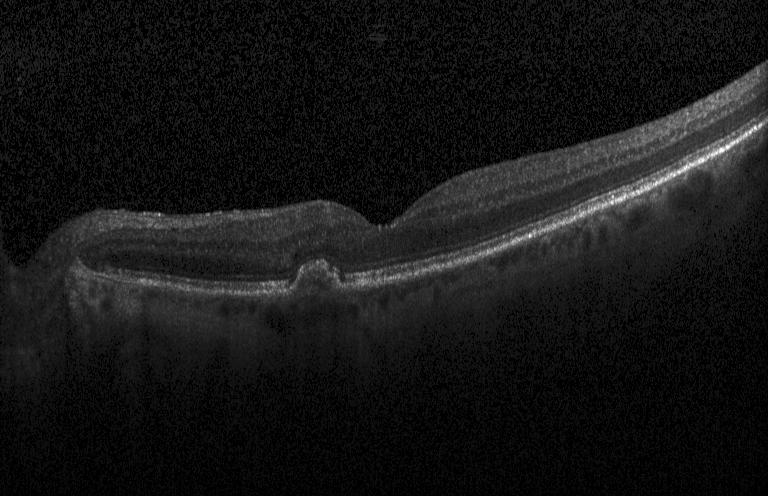 Through the macula; Heidelberg Spectralis OCT system; spectral-domain optical coherence tomography; OCT line scan — Impression: a choroidal neovascular membrane.